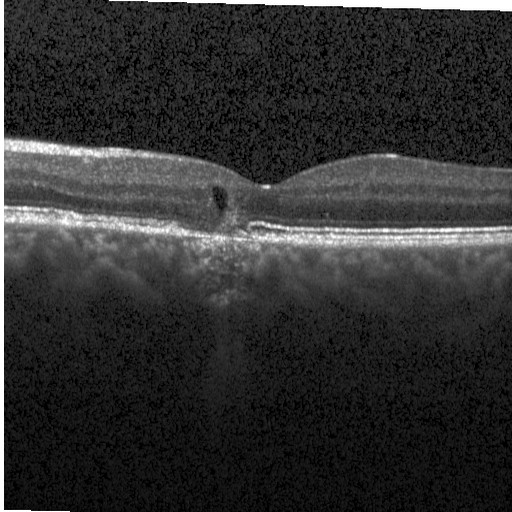 Diagnosis: DME.